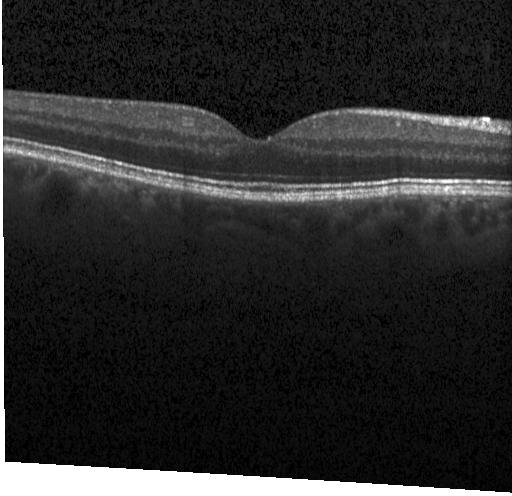
OCT line scan; centered on the fovea; Heidelberg Spectralis; SD-OCT.
Finding: no choroidal neovascularization, diabetic macular edema, or drusen.